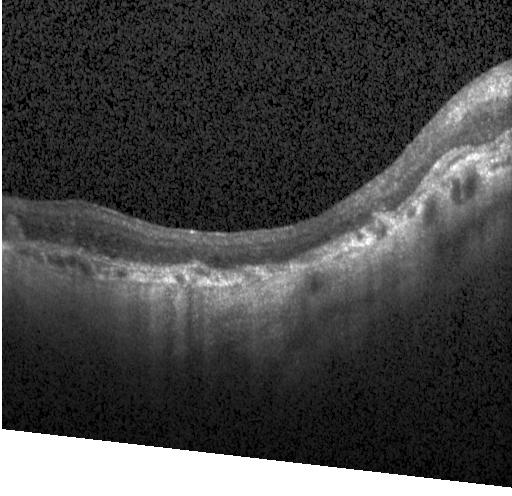
SD-OCT; retinal OCT cross-section; acquired on a Heidelberg Spectralis
This B-scan demonstrates CNV.